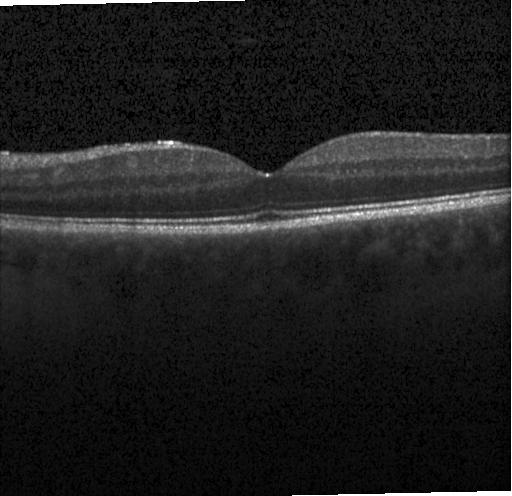
Assessment: no evidence of choroidal neovascularization, diabetic macular edema, or drusen.